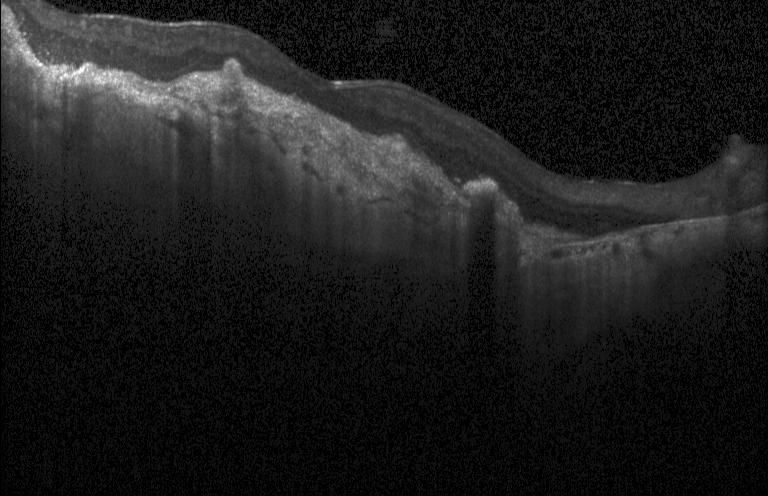
Spectral-domain OCT, optical coherence tomography scan, through the macula, Heidelberg Spectralis — Dx: choroidal neovascularization (CNV).